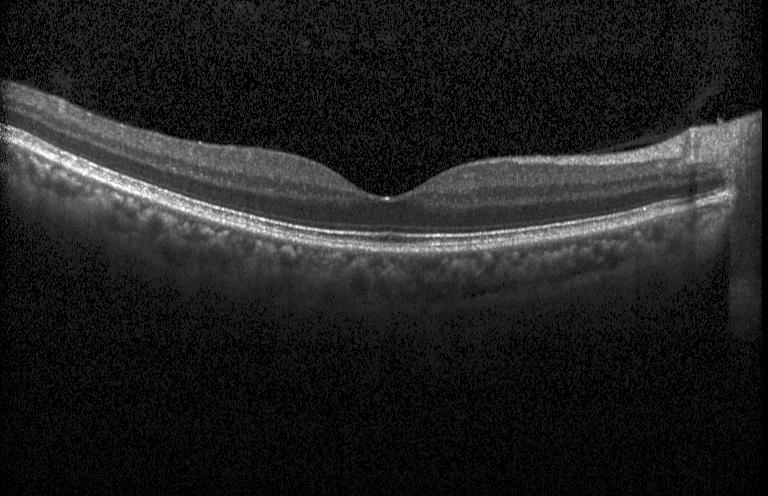 Instrument: Heidelberg Spectralis. Spectral-domain OCT. Retinal OCT cross-section. Through the macula.
Impression: no evidence of choroidal neovascularization, diabetic macular edema, or drusen.